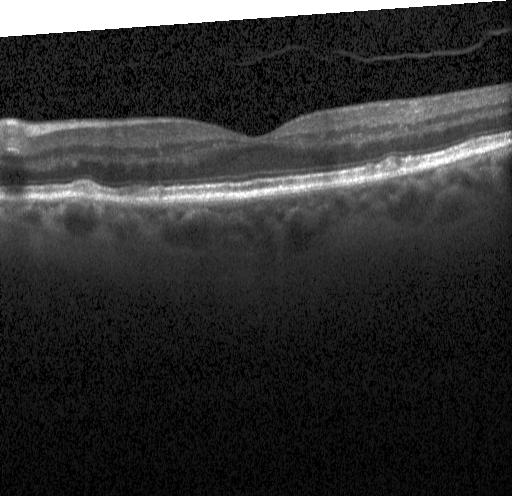 OCT line scan
Diagnosis: sub-RPE drusenoid deposits.